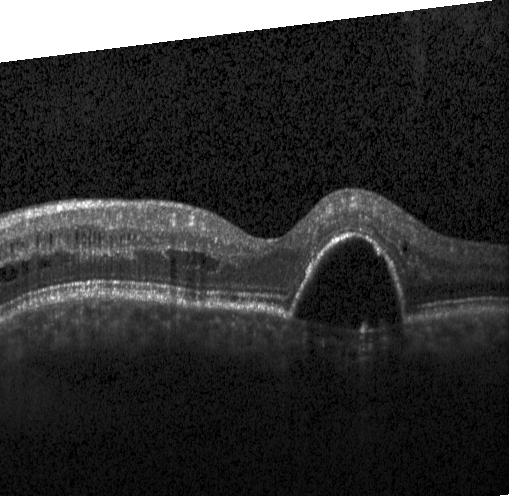
Retinal OCT cross-section · acquired on a Heidelberg Spectralis
This B-scan demonstrates a choroidal neovascular membrane.